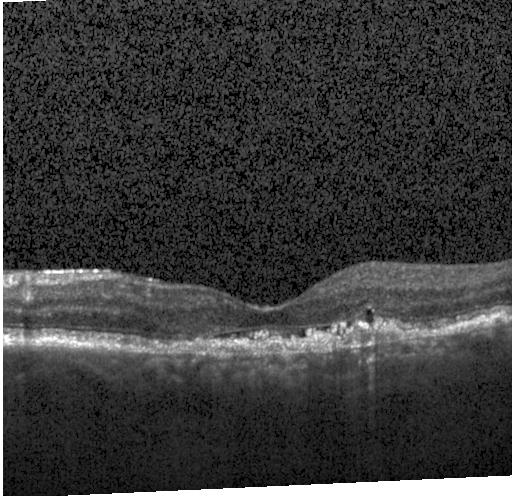 Macular scan · retinal OCT cross-section · SD-OCT
Finding: a choroidal neovascular membrane.